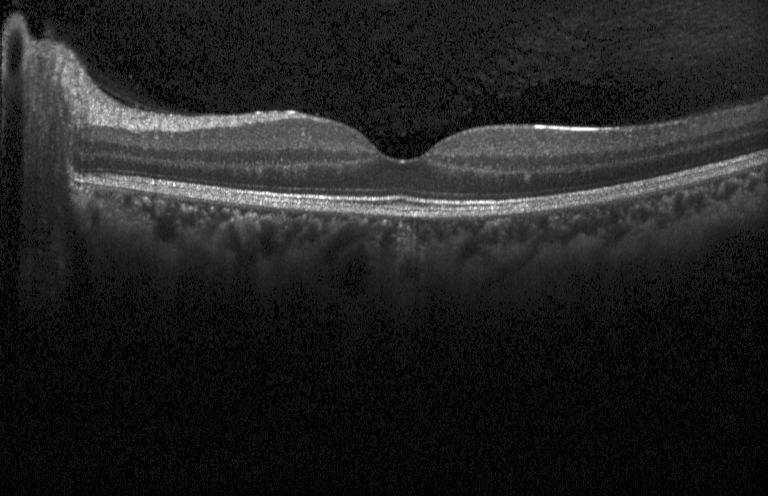
Retinal OCT B-scan · acquired on a Heidelberg Spectralis · horizontal scan through the fovea.
Diagnosis: neither choroidal neovascularization, diabetic macular edema, nor drusen.